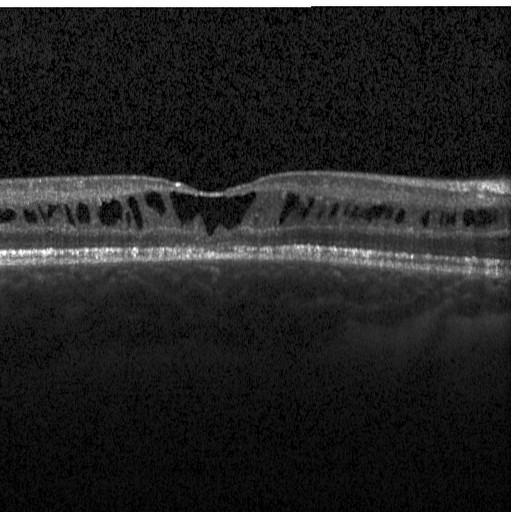 Finding: DME.